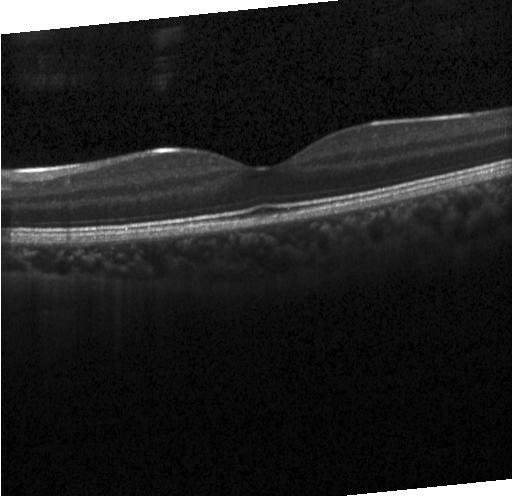 Retinal OCT cross-section showing no choroidal neovascularization, diabetic macular edema, or drusen.